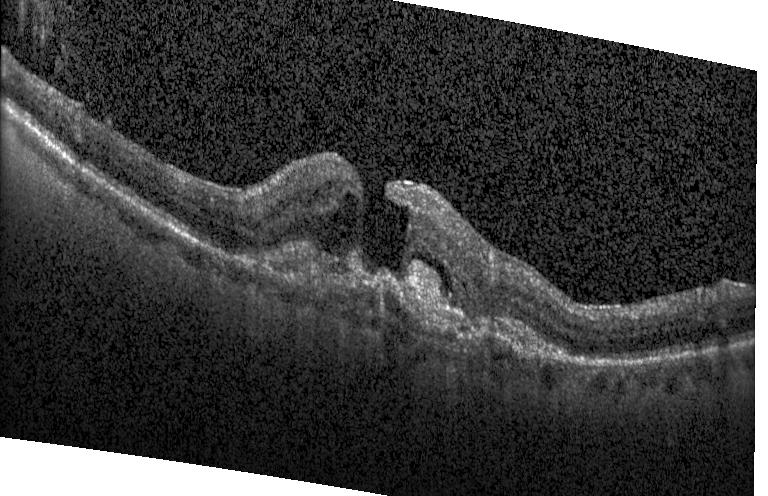

Diagnosis: choroidal neovascularization (CNV).